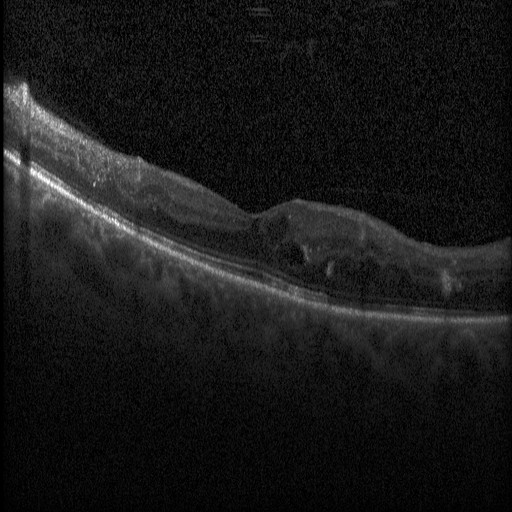 Retinal OCT cross-section showing diabetic macular edema (DME).